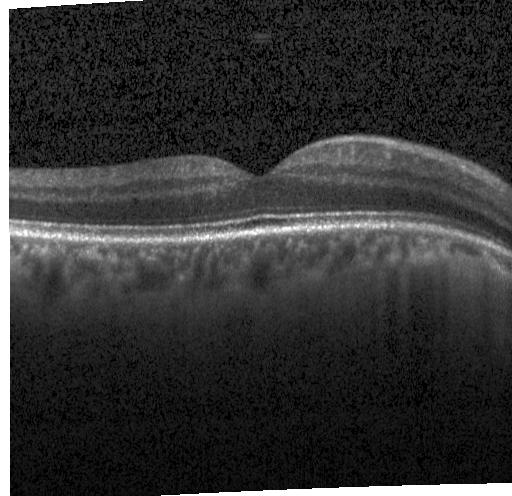
Diagnosis: no evidence of CNV, DME, or drusen.